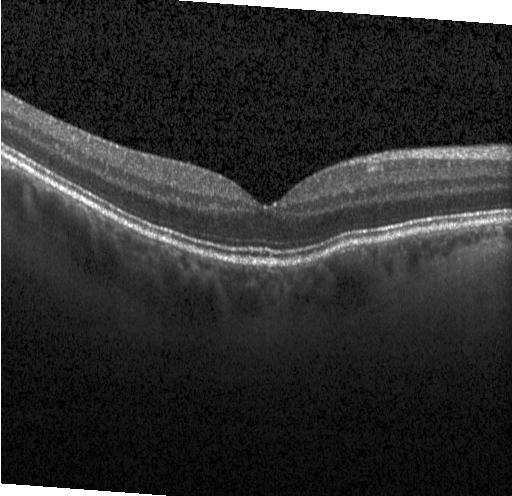
Optical coherence tomography B-scan; Heidelberg Spectralis OCT system. The scan shows no evidence of choroidal neovascularization, diabetic macular edema, or drusen.